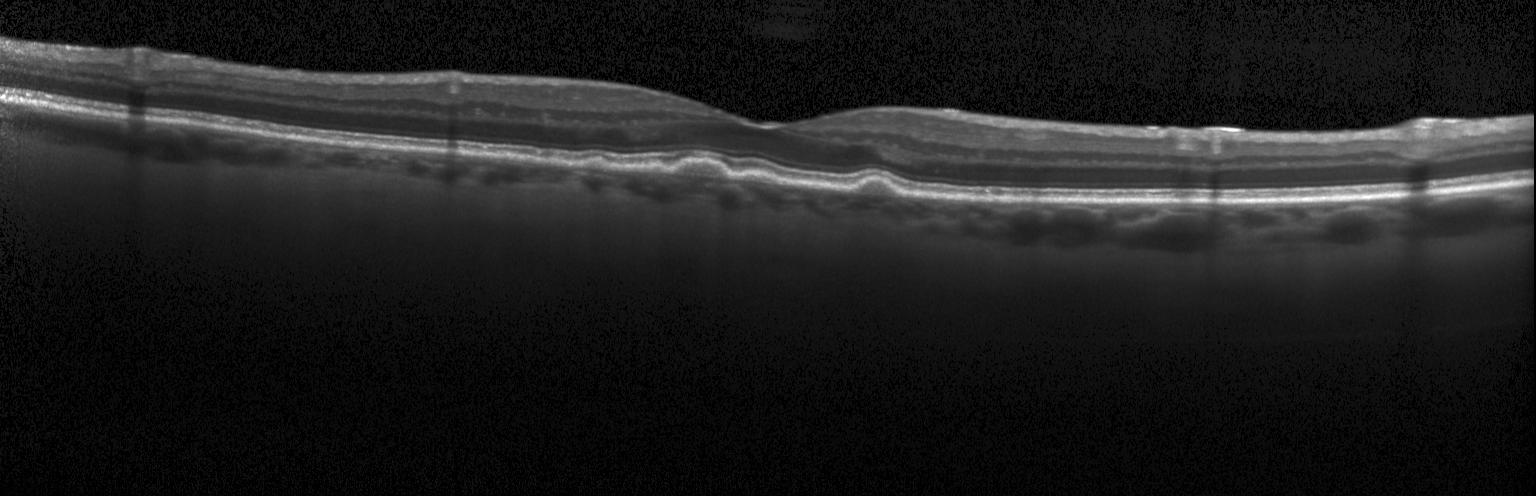 Horizontal scan through the fovea · OCT B-scan. Diagnosis: multiple drusen.